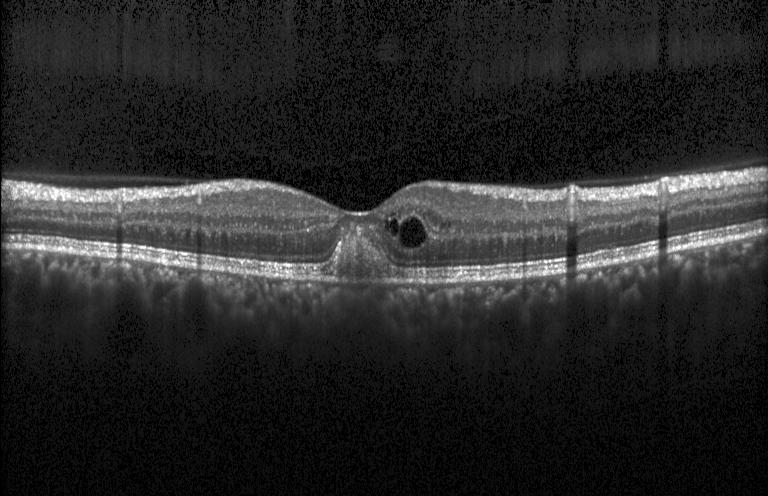 Instrument: Heidelberg Spectralis; retinal OCT B-scan; fovea-centered — This B-scan demonstrates a choroidal neovascular membrane.